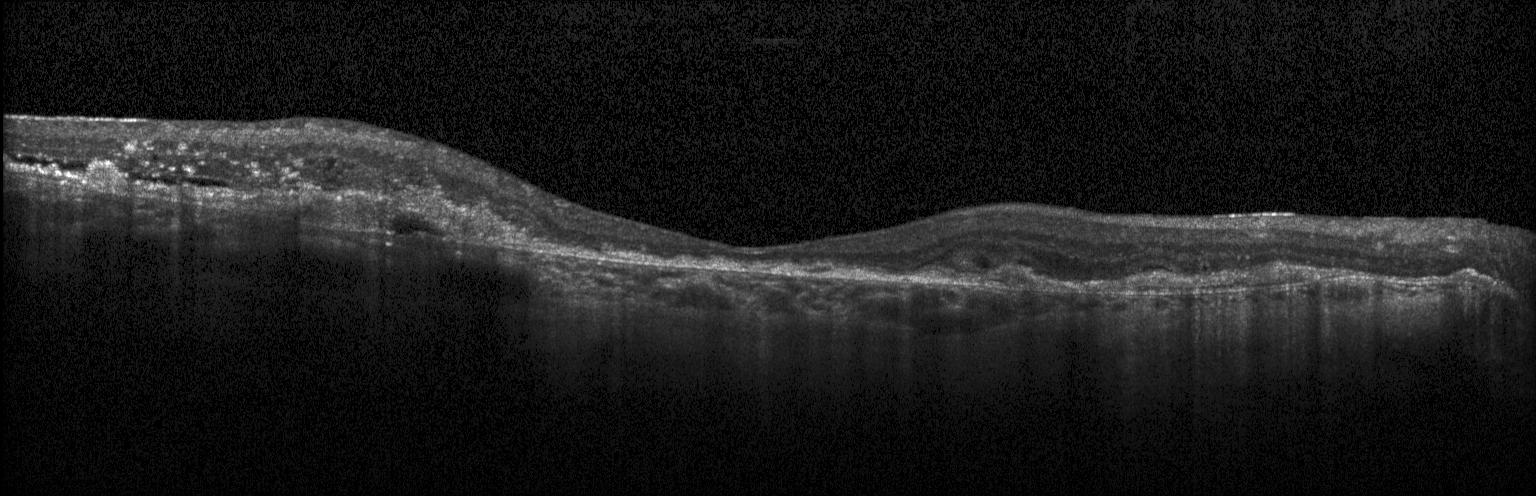 OCT scan showing a choroidal neovascular membrane.